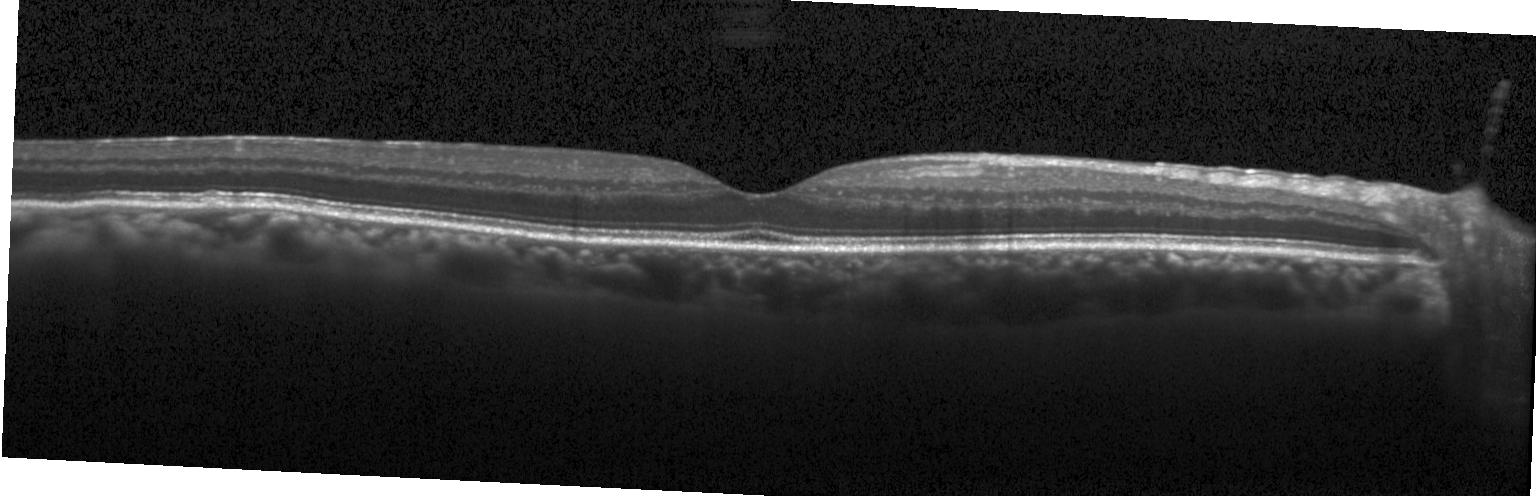
Acquired on a Heidelberg Spectralis. OCT B-scan. Fovea-centered. OCT finding: neither choroidal neovascularization, diabetic macular edema, nor drusen.